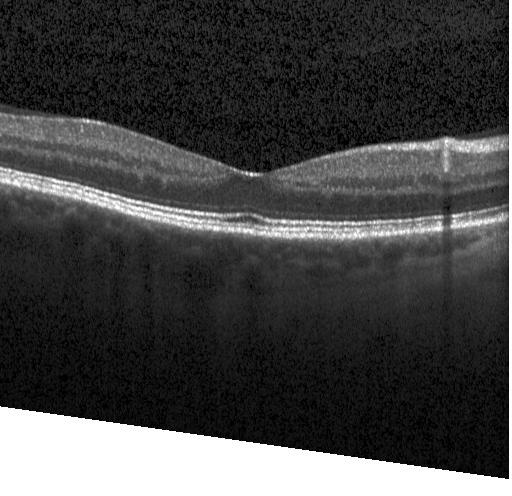

Spectral-domain OCT B-scan: no CNV, no DME, and no drusen.